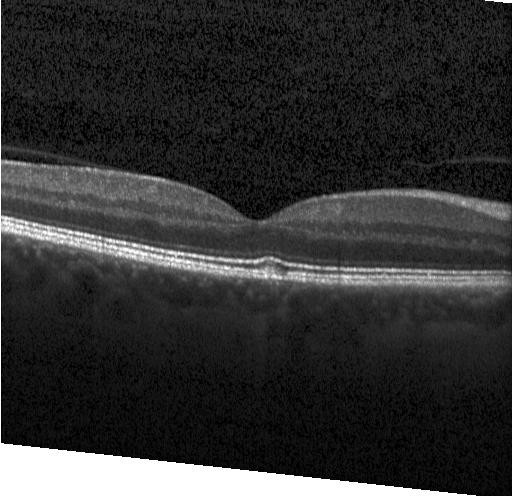
Acquired on a Heidelberg Spectralis; horizontal scan through the fovea; retinal OCT B-scan.
Assessment: neither choroidal neovascularization, diabetic macular edema, nor drusen.